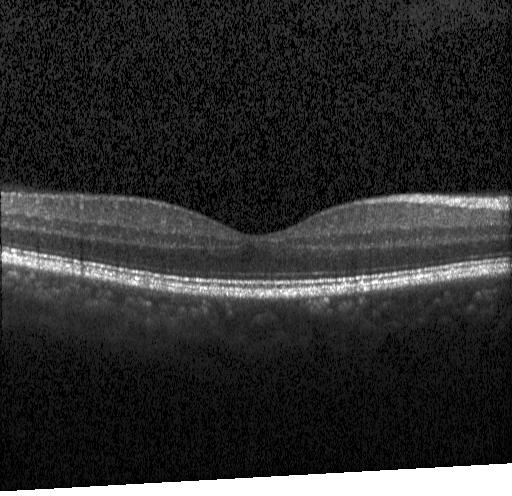

SD-OCT, through the macula, retinal OCT cross-section — Impression: no choroidal neovascularization, diabetic macular edema, or drusen.